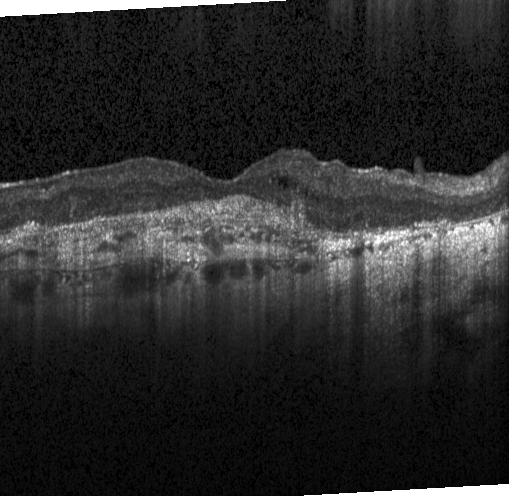

OCT finding: choroidal neovascularization.